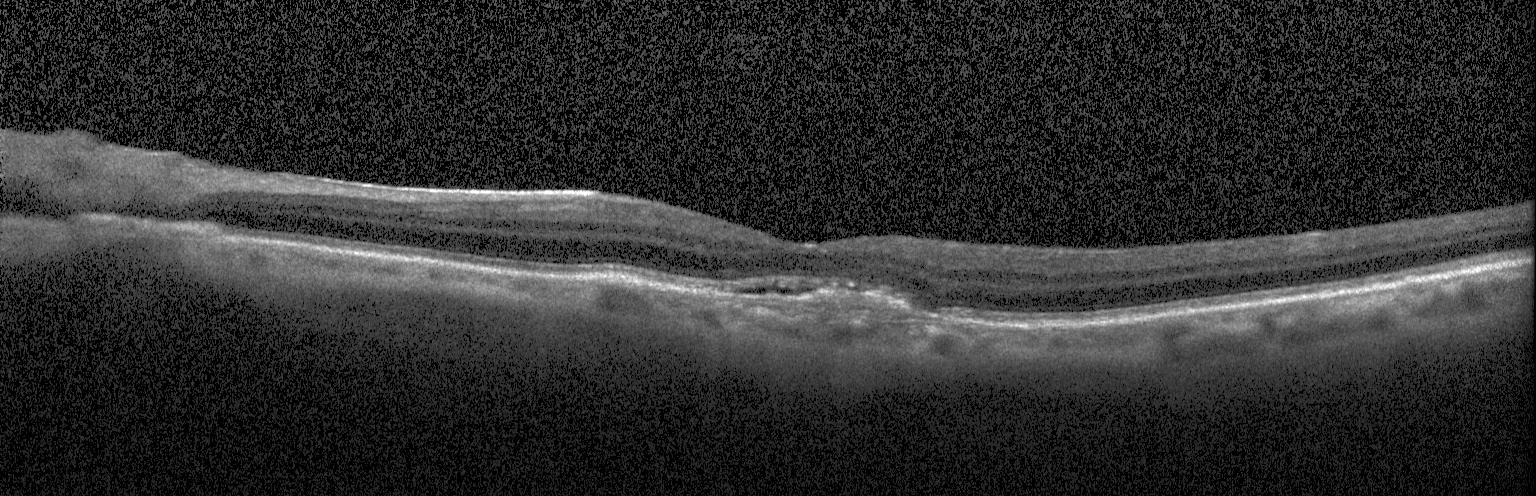 Optical coherence tomography B-scan. Heidelberg Spectralis. Spectral-domain OCT — Impression: a choroidal neovascular membrane.